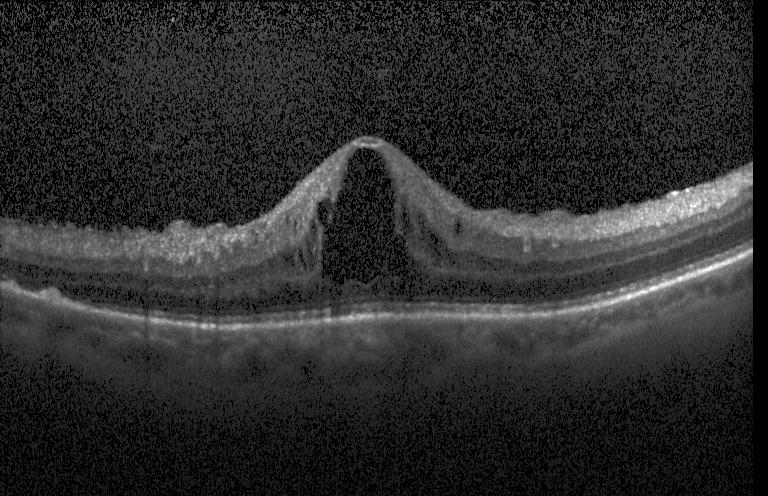

OCT B-scan showing diabetic macular edema (DME).